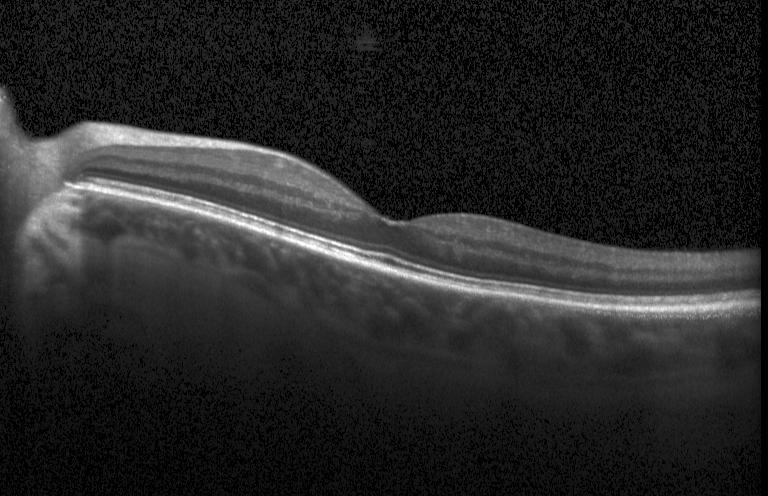 OCT scan showing no choroidal neovascularization, no diabetic macular edema, and no drusen.